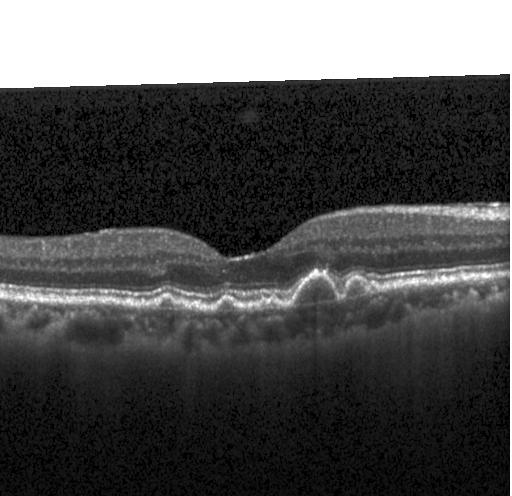

OCT finding: sub-RPE drusenoid deposits.